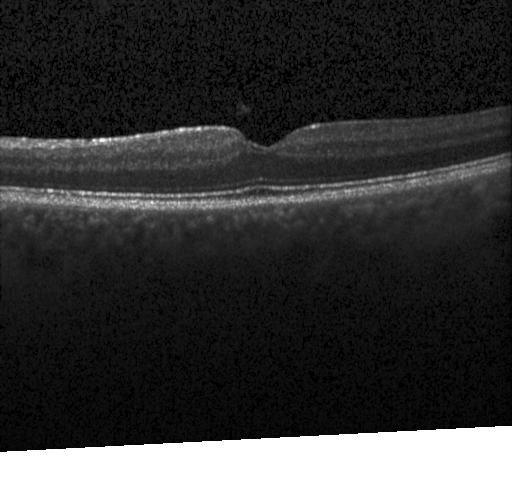

Spectral-domain optical coherence tomography. Macular scan. Optical coherence tomography scan. Heidelberg Spectralis OCT system.
Dx: no choroidal neovascularization, no diabetic macular edema, and no drusen.